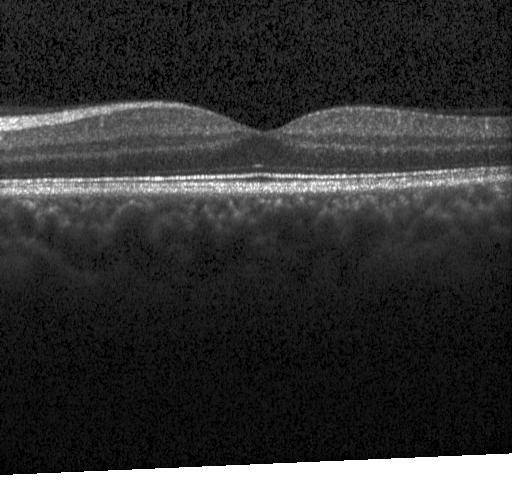

SD-OCT; optical coherence tomography scan; macular scan — The scan shows neither choroidal neovascularization, diabetic macular edema, nor drusen.